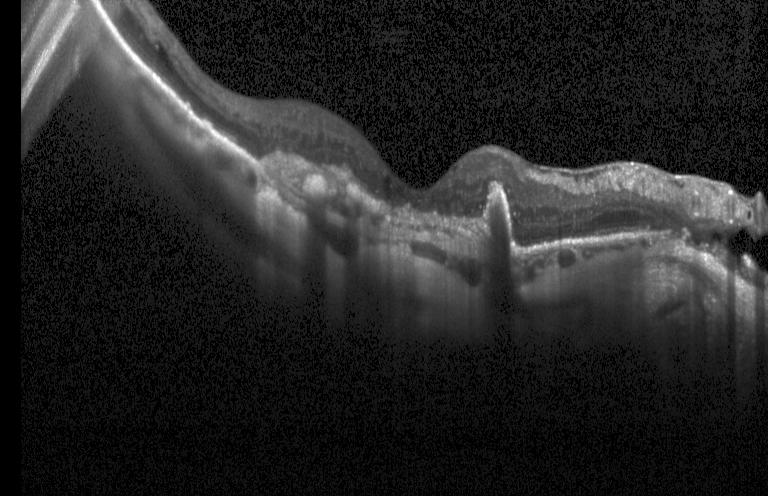

Heidelberg Spectralis; horizontal scan through the fovea; spectral-domain OCT; optical coherence tomography B-scan.
This B-scan demonstrates a choroidal neovascular membrane.